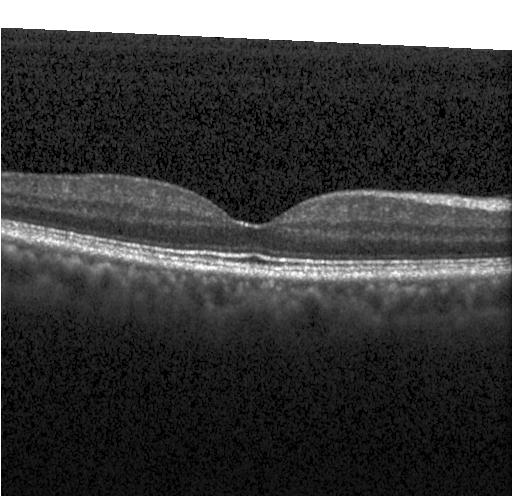 Optical coherence tomography B-scan. Macular OCT: no evidence of choroidal neovascularization, diabetic macular edema, or drusen.